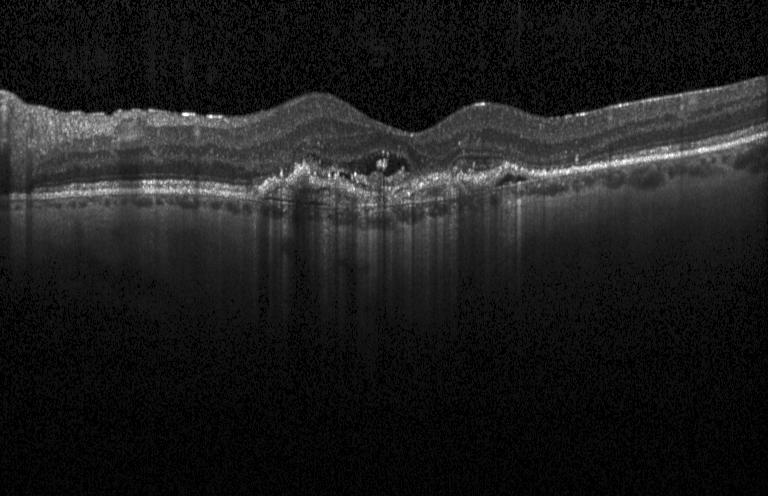
Fovea-centered · optical coherence tomography B-scan
Choroidal neovascularization (CNV).